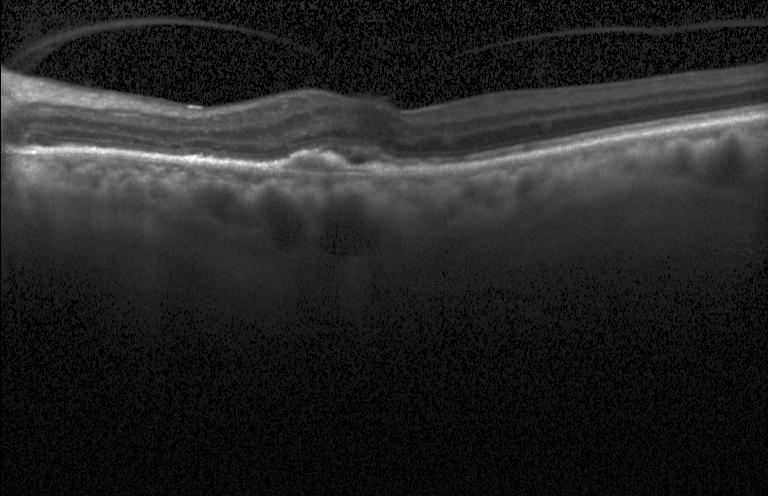
OCT B-scan showing a choroidal neovascular membrane.